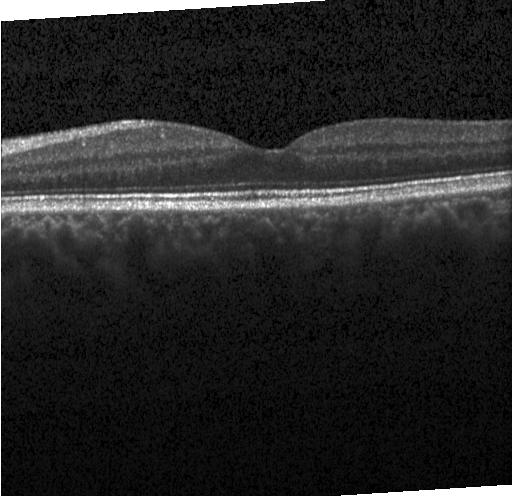 Impression: no choroidal neovascularization, diabetic macular edema, or drusen.